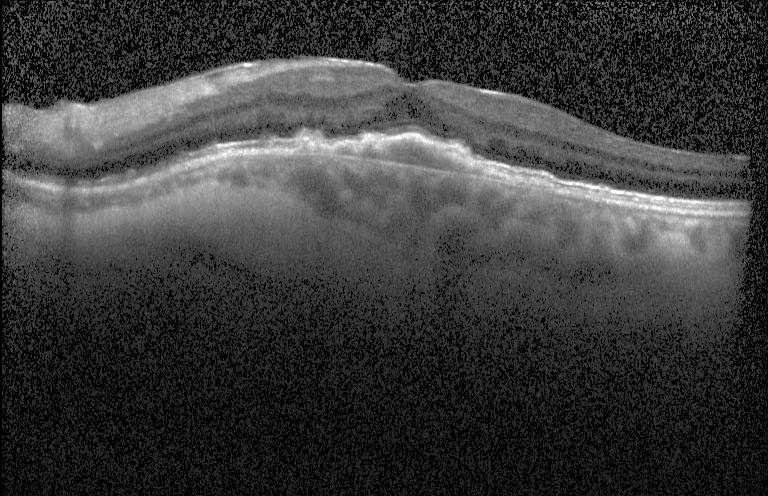
Horizontal scan through the fovea. Heidelberg Spectralis. Optical coherence tomography scan — This B-scan demonstrates choroidal neovascularization (CNV).